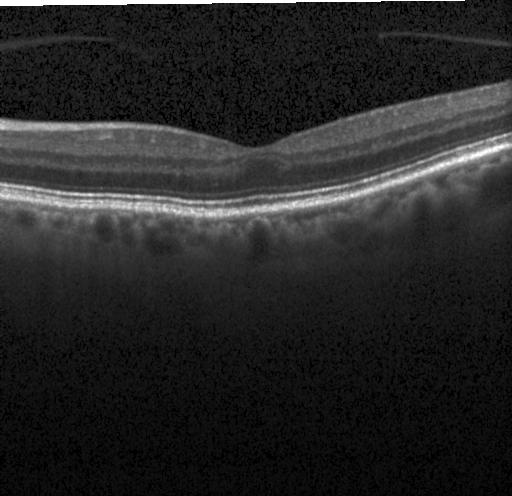 Heidelberg Spectralis OCT system · optical coherence tomography B-scan · spectral-domain OCT
Impression: neither CNV, DME, nor drusen.